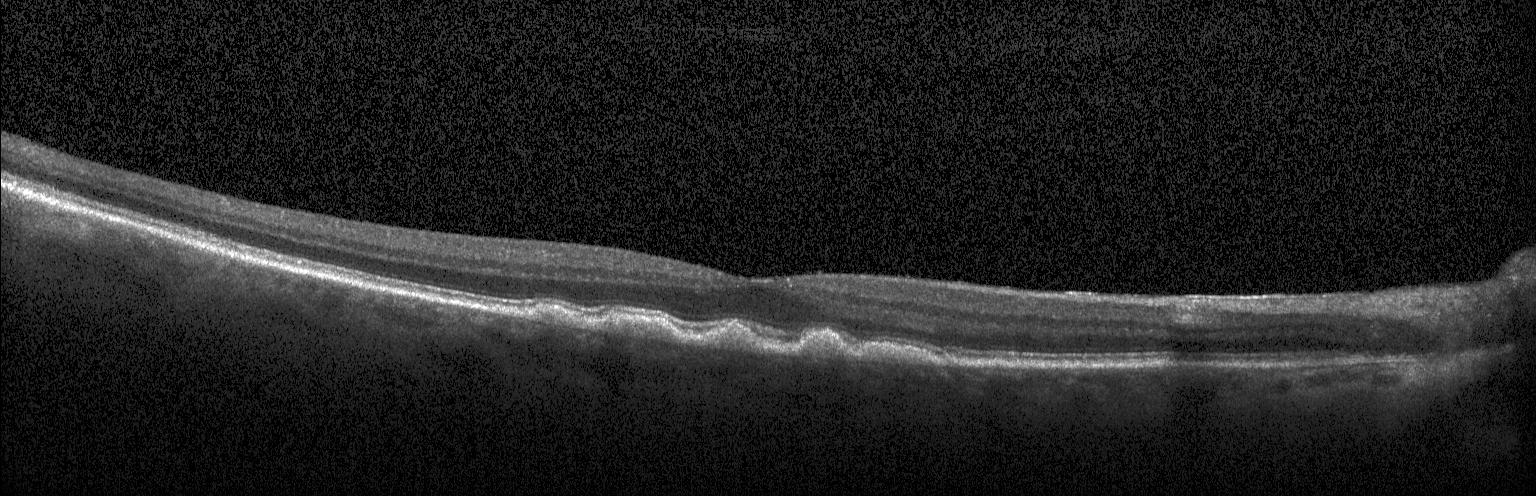 Finding: multiple drusen.